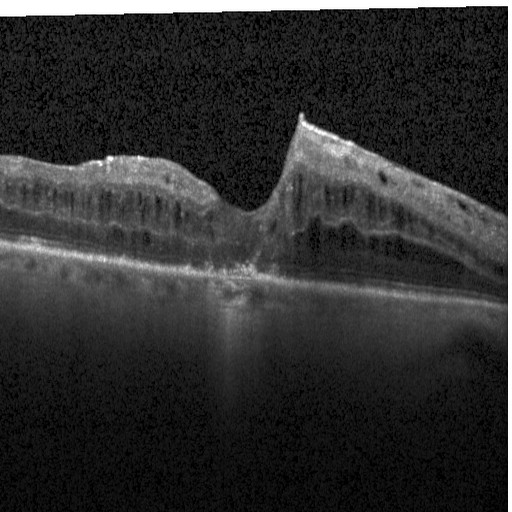 Retinal OCT B-scan, centered on the fovea.
Impression: DME.